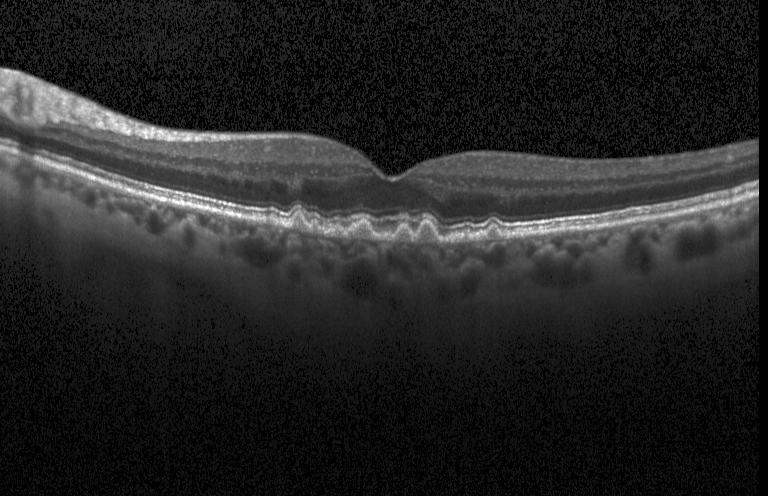 Retinal OCT cross-section showing sub-RPE drusenoid deposits.